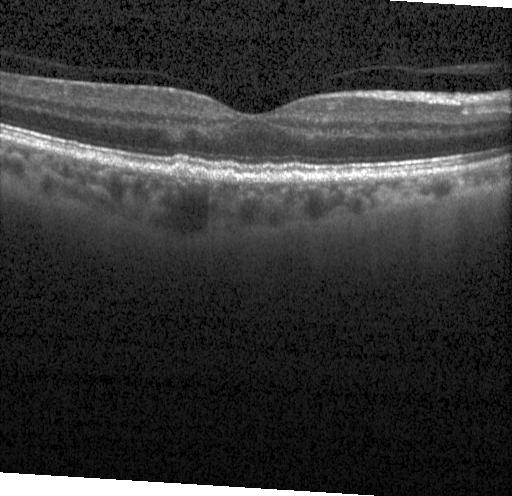
Assessment: drusen.